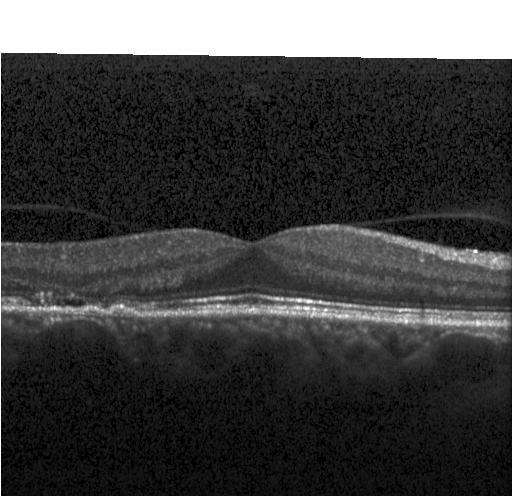

Spectral-domain OCT. Horizontal scan through the fovea. Retinal OCT cross-section. Heidelberg Spectralis
A choroidal neovascular membrane.